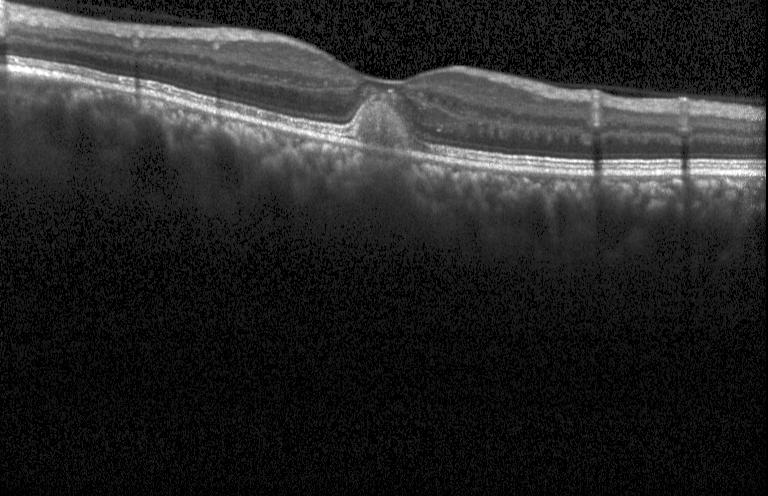

Retinal OCT cross-section · Heidelberg Spectralis OCT system · spectral-domain optical coherence tomography — Diagnosis: CNV.